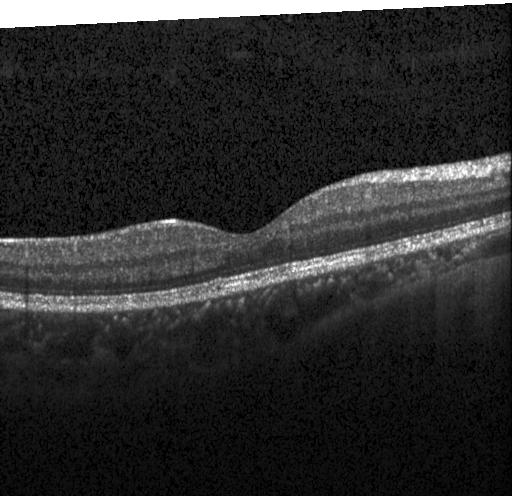
This B-scan demonstrates no choroidal neovascularization, no diabetic macular edema, and no drusen.